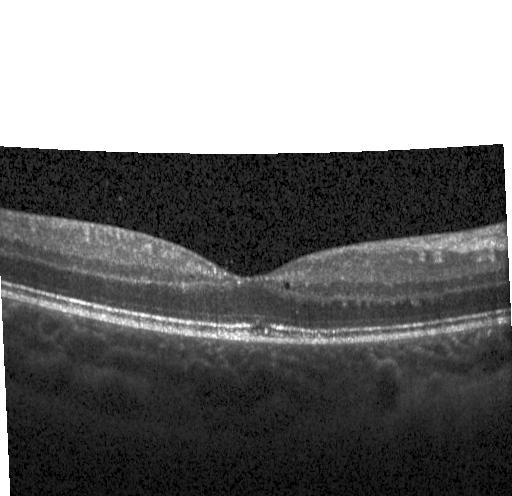 Retinal OCT B-scan, spectral-domain OCT
Diagnosis: diabetic macular edema (DME).